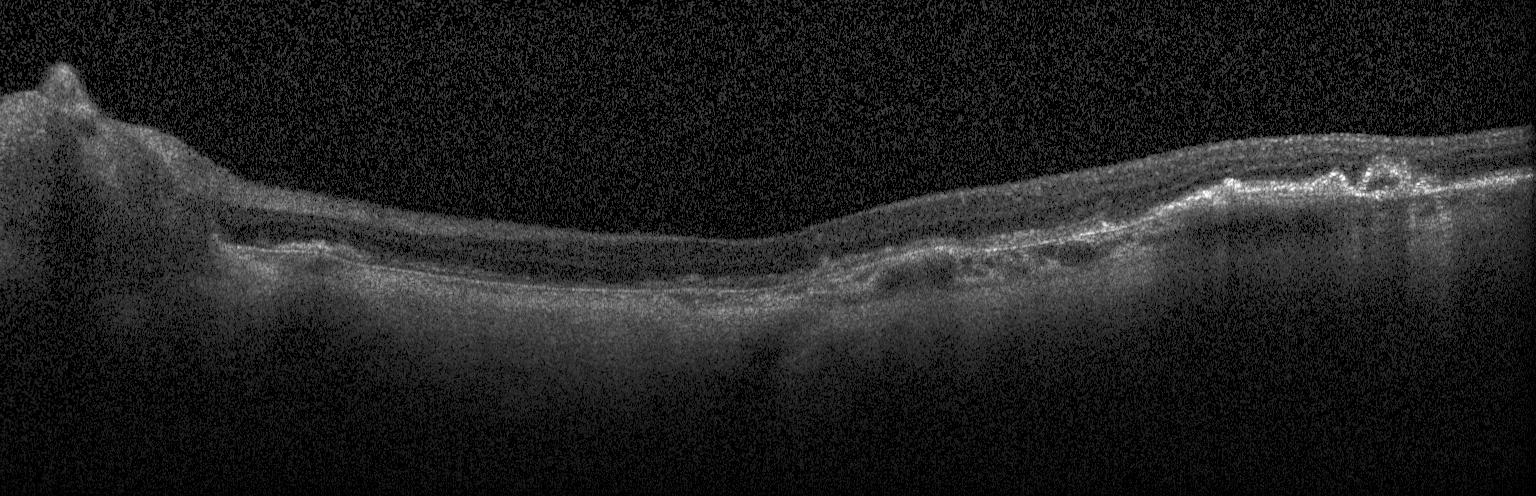 Impression: choroidal neovascularization.